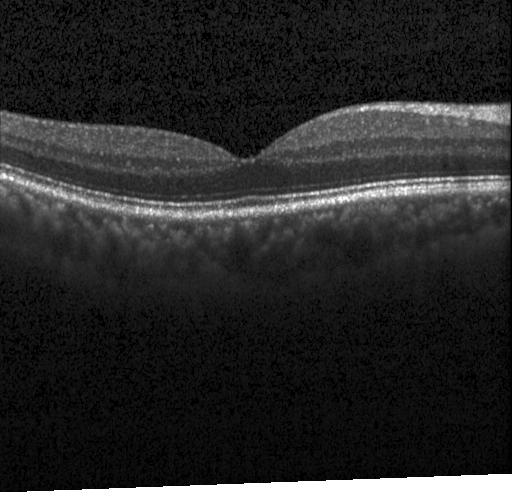

Spectral-domain OCT B-scan: no evidence of CNV, DME, or drusen.